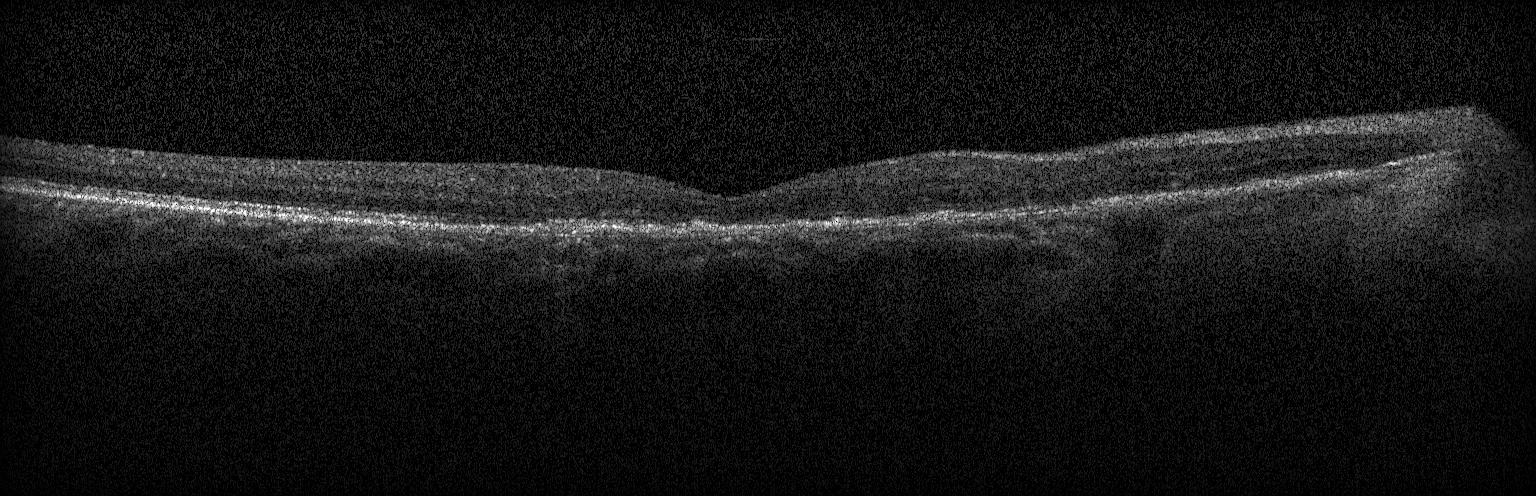

Optical coherence tomography scan
Impression: choroidal neovascularization (CNV).